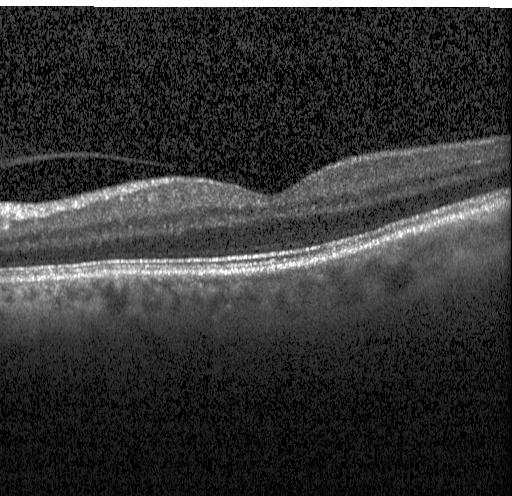
Heidelberg Spectralis OCT system, optical coherence tomography B-scan, macular scan
Macular OCT: no evidence of choroidal neovascularization, diabetic macular edema, or drusen.